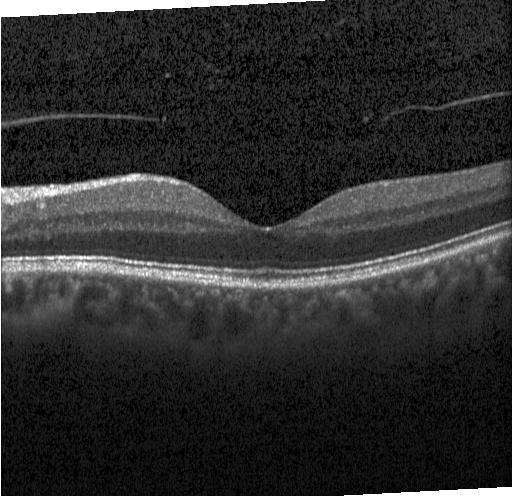 Spectral-domain optical coherence tomography; Heidelberg Spectralis; retinal OCT B-scan
The scan shows no choroidal neovascularization, diabetic macular edema, or drusen.